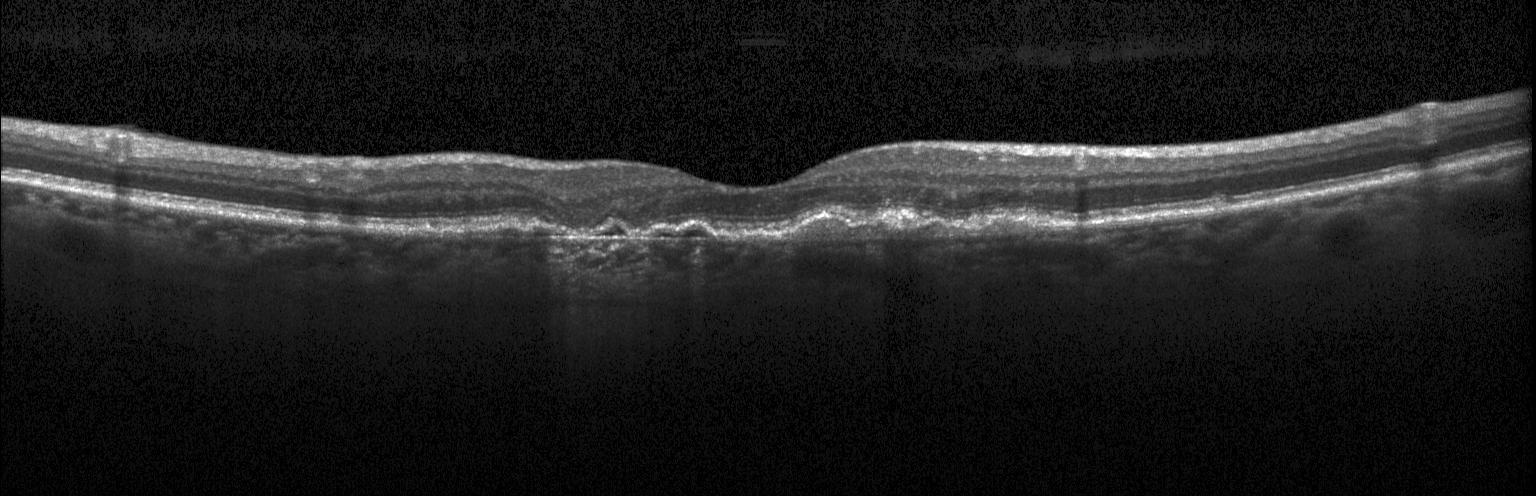

Macular scan. Retinal OCT cross-section. SD-OCT. Heidelberg Spectralis OCT system
Diagnosis: choroidal neovascularization.